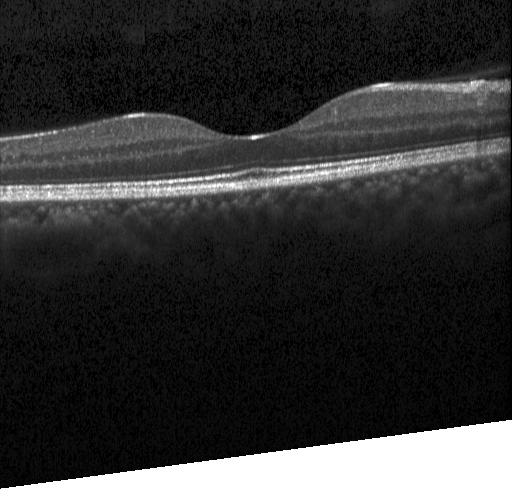 Instrument: Heidelberg Spectralis, SD-OCT, optical coherence tomography scan.
Impression: neither choroidal neovascularization, diabetic macular edema, nor drusen.